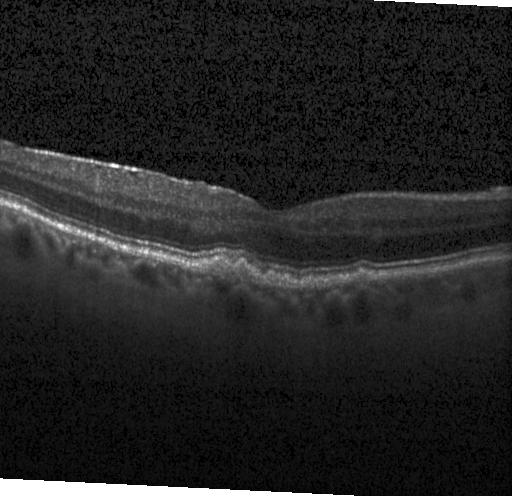 Retinal OCT B-scan
Macular OCT: multiple drusen.